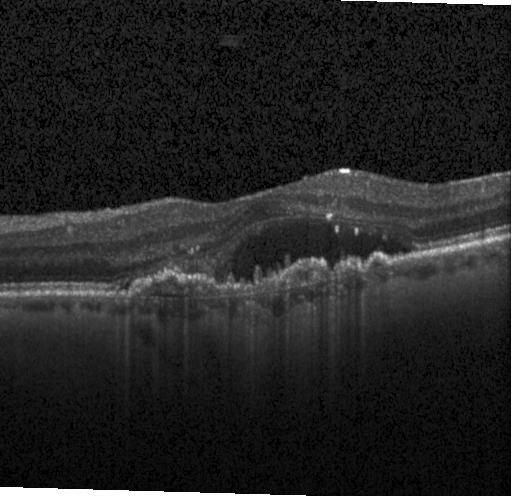
The scan shows a choroidal neovascular membrane.